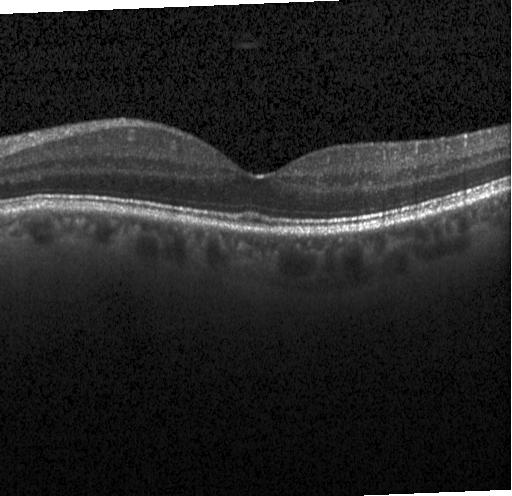
Retinal OCT cross-section — Assessment: no choroidal neovascularization, no diabetic macular edema, and no drusen.